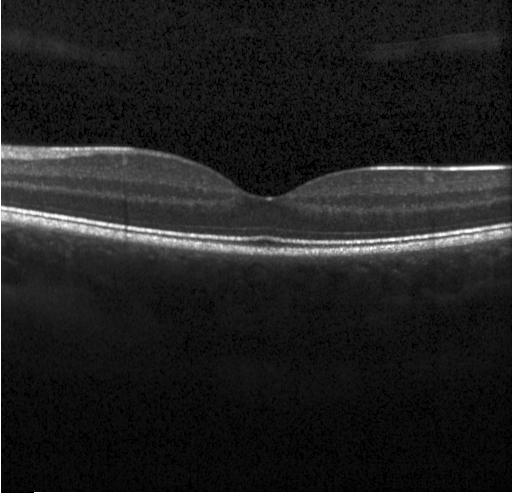
OCT line scan, instrument: Heidelberg Spectralis, SD-OCT — Finding: no evidence of choroidal neovascularization, diabetic macular edema, or drusen.